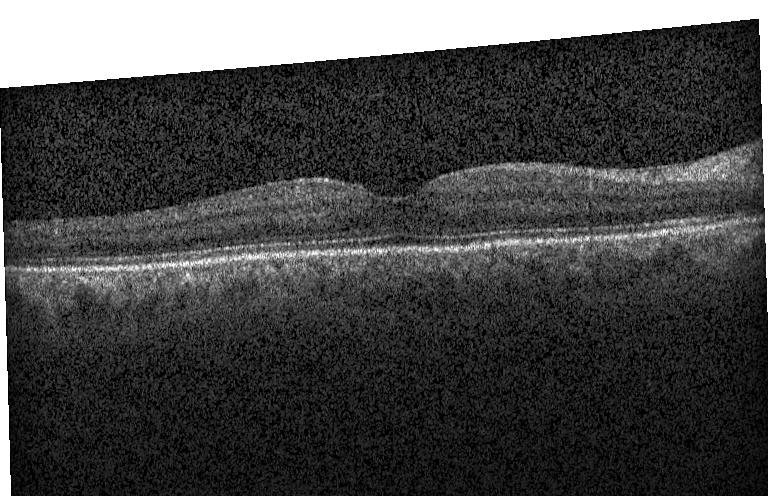

Spectral-domain OCT B-scan: neither CNV, DME, nor drusen.